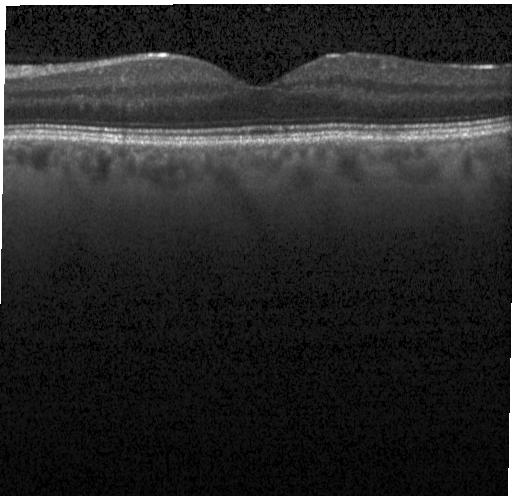

Instrument: Heidelberg Spectralis · OCT line scan.
Finding: no choroidal neovascularization, no diabetic macular edema, and no drusen.